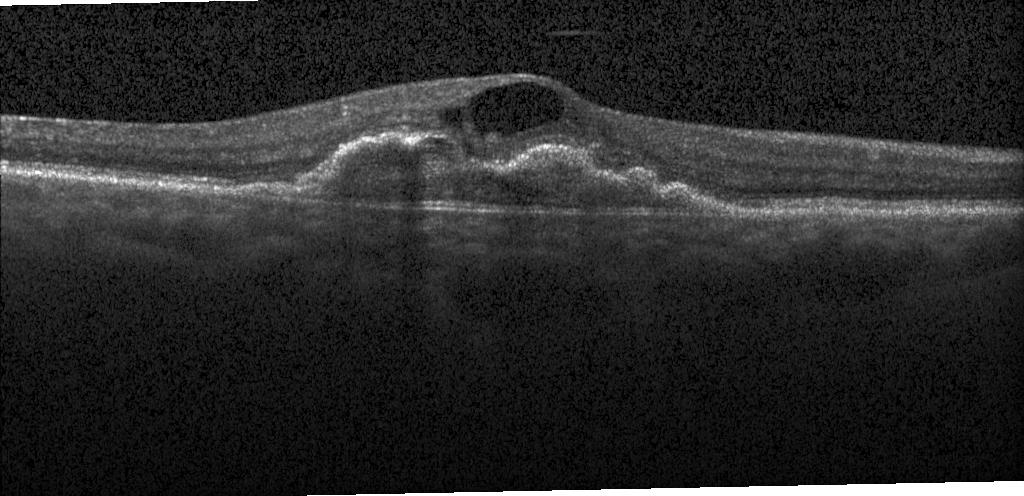 Optical coherence tomography scan. Spectral-domain optical coherence tomography. Finding: choroidal neovascularization (CNV).